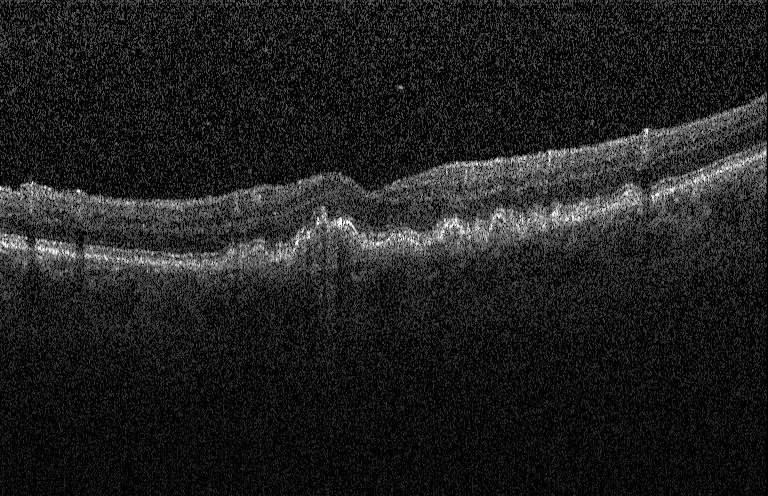

OCT line scan.
This B-scan demonstrates a choroidal neovascular membrane.